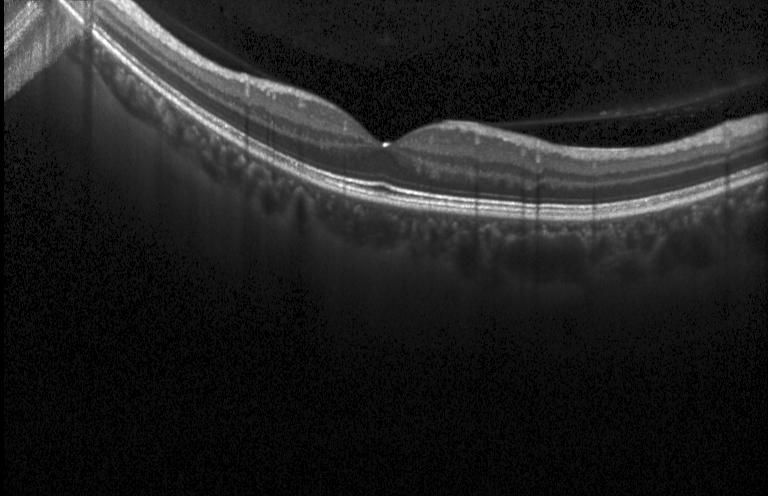

OCT finding: no CNV, no DME, and no drusen.